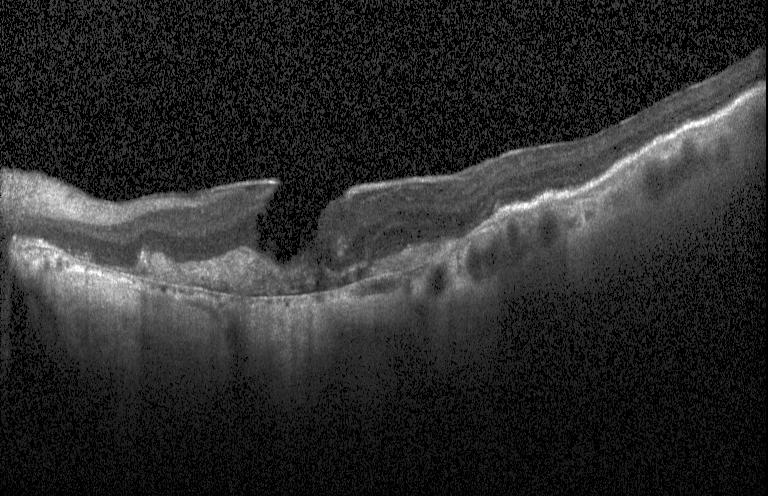 The scan shows choroidal neovascularization.